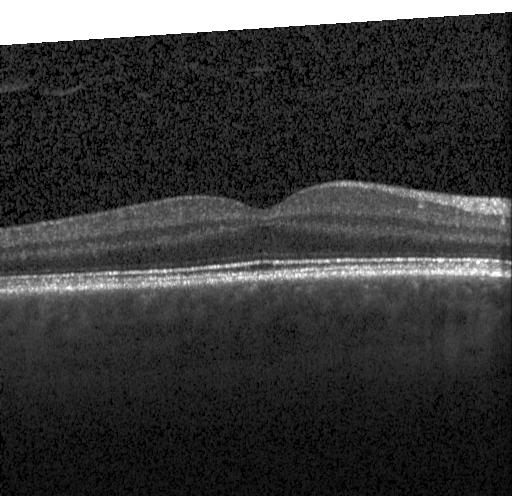 OCT line scan, spectral-domain optical coherence tomography, Heidelberg Spectralis
Impression: no CNV, no DME, and no drusen.